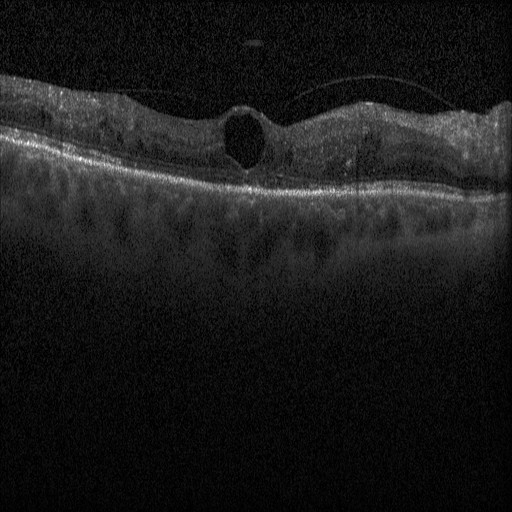

Macular scan · retinal OCT B-scan · SD-OCT.
Diagnosis: DME.